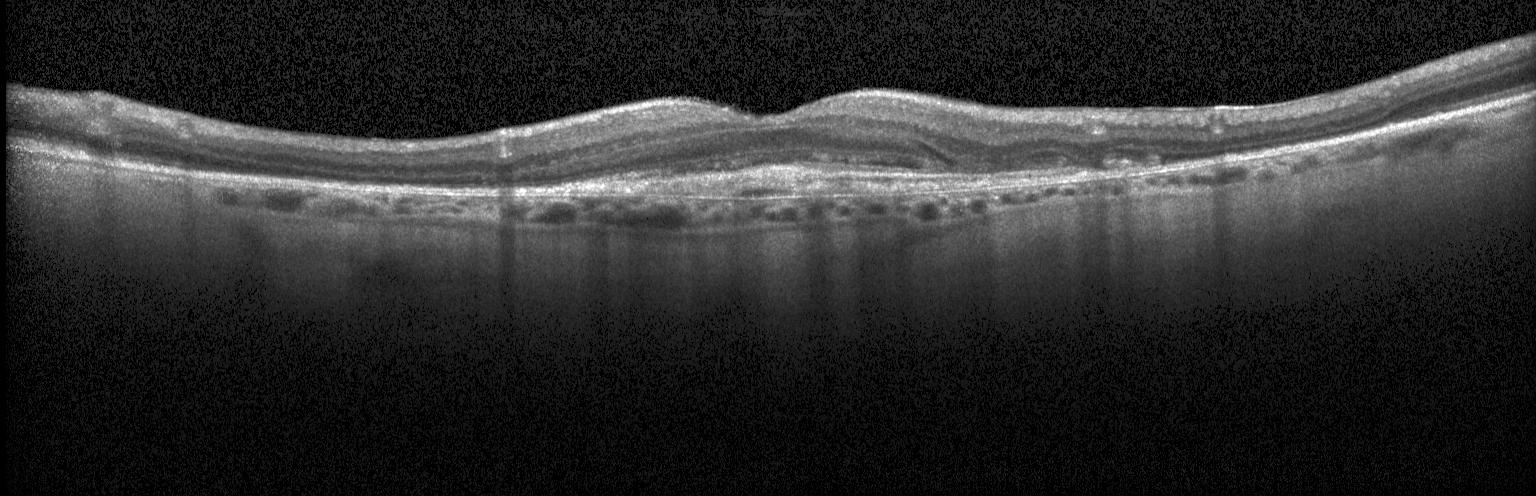

OCT B-scan. Spectral-domain OCT. Instrument: Heidelberg Spectralis. Assessment: choroidal neovascularization.